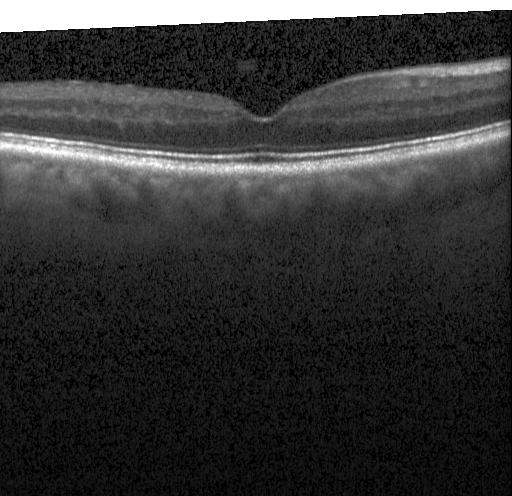 Retinal OCT B-scan · instrument: Heidelberg Spectralis · spectral-domain OCT — Assessment: no choroidal neovascularization, diabetic macular edema, or drusen.